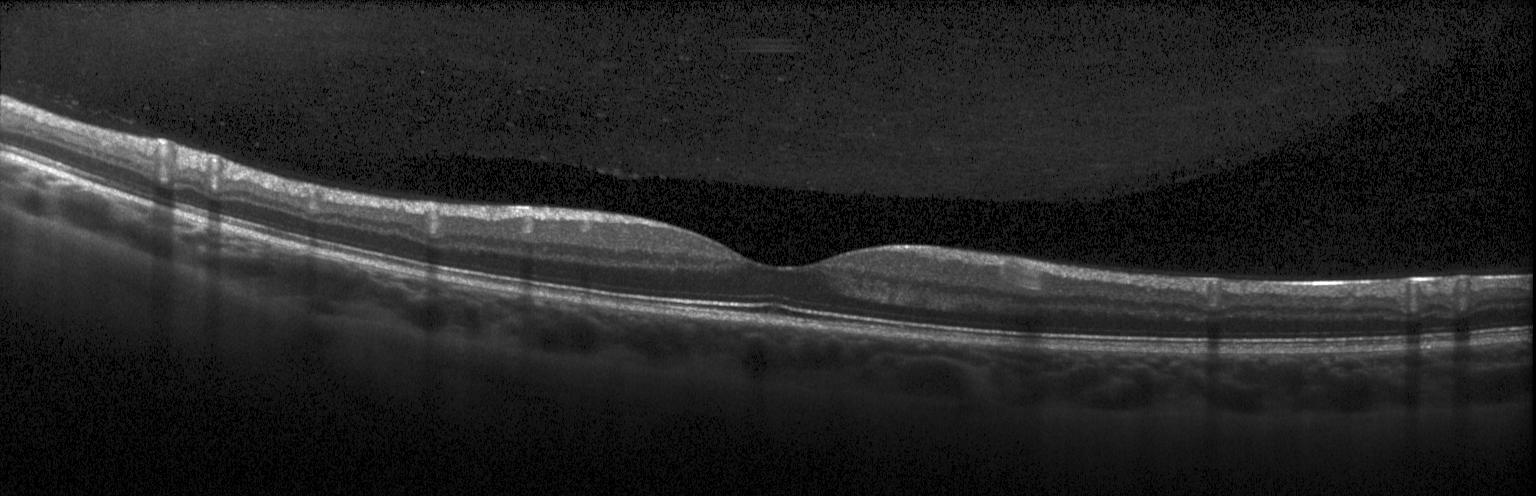

Assessment: no choroidal neovascularization, diabetic macular edema, or drusen.